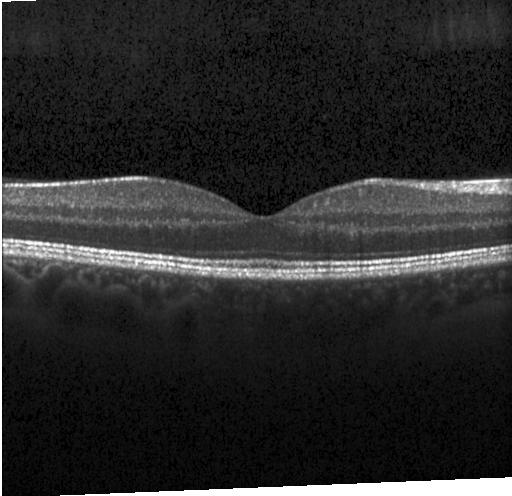

OCT B-scan · acquired on a Heidelberg Spectralis · through the macula
Finding: no evidence of choroidal neovascularization, diabetic macular edema, or drusen.